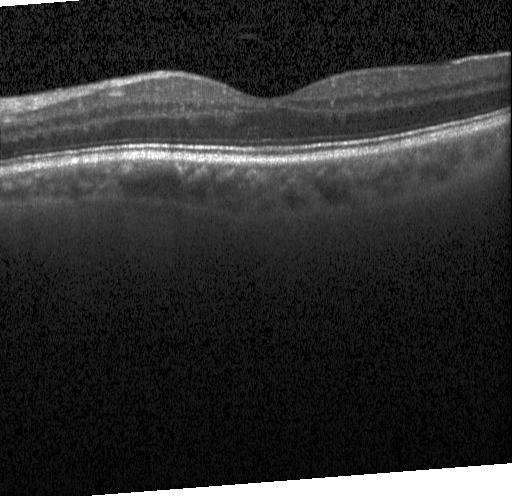

Spectral-domain OCT · retinal OCT cross-section · Heidelberg Spectralis · centered on the fovea — Impression: neither CNV, DME, nor drusen.